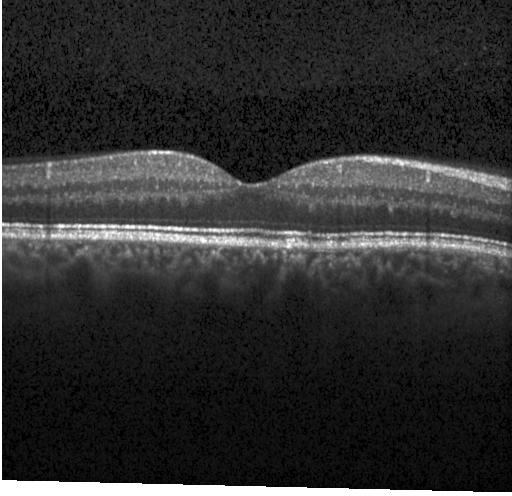
SD-OCT, instrument: Heidelberg Spectralis, retinal OCT cross-section
Diagnosis: no evidence of CNV, DME, or drusen.